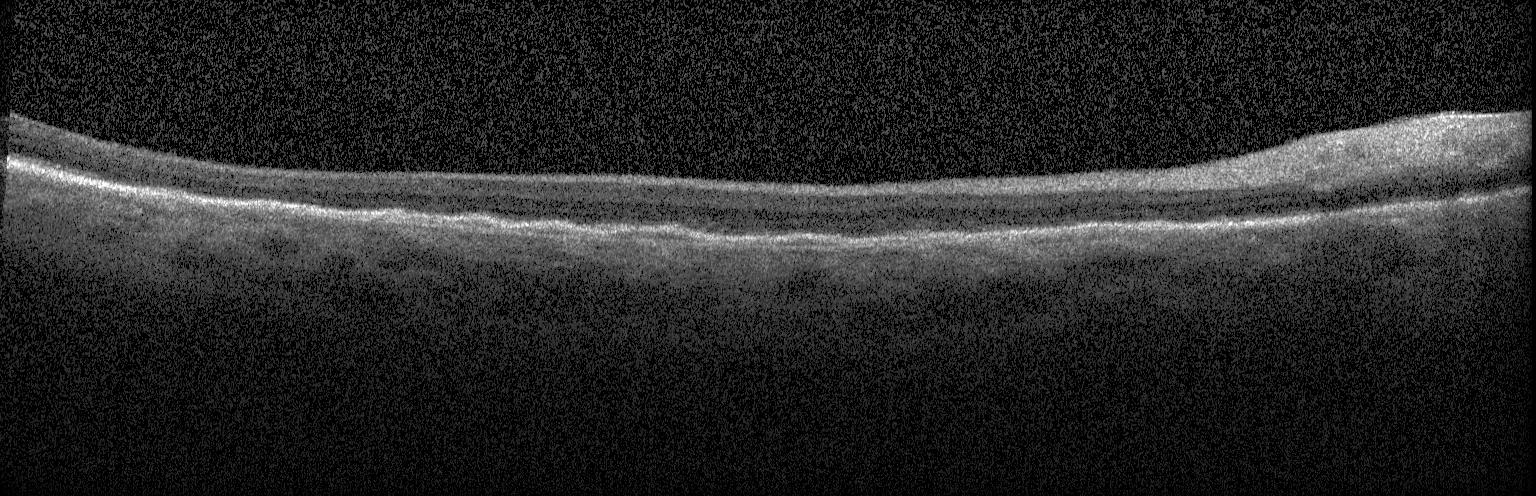
OCT B-scan showing a choroidal neovascular membrane.